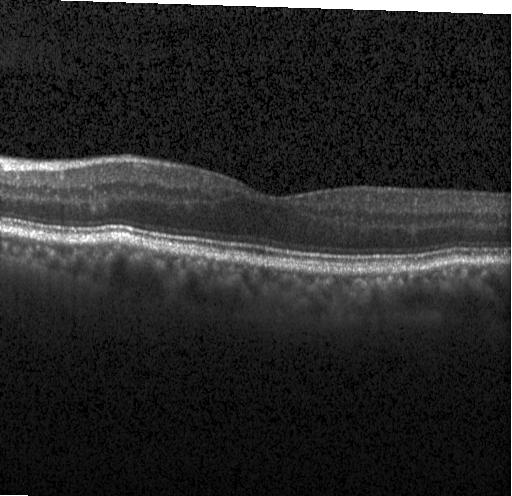
Optical coherence tomography scan, SD-OCT, centered on the fovea, instrument: Heidelberg Spectralis.
Diagnosis: no evidence of choroidal neovascularization, diabetic macular edema, or drusen.